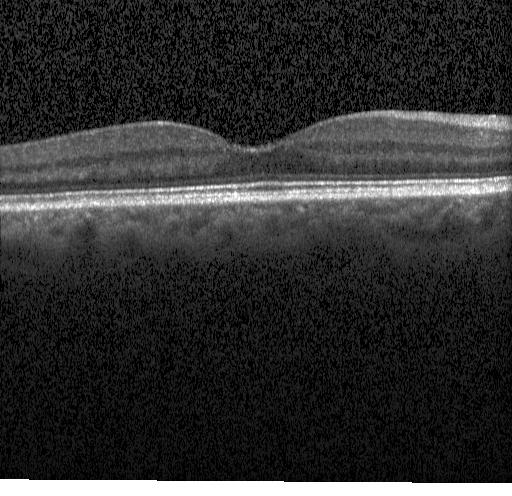

OCT scan showing no evidence of CNV, DME, or drusen.